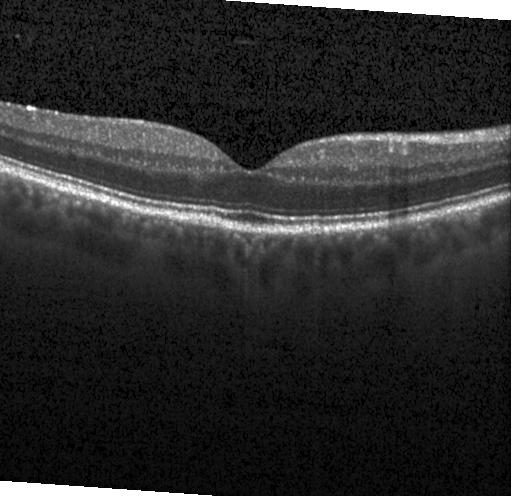
Finding: no choroidal neovascularization, no diabetic macular edema, and no drusen.